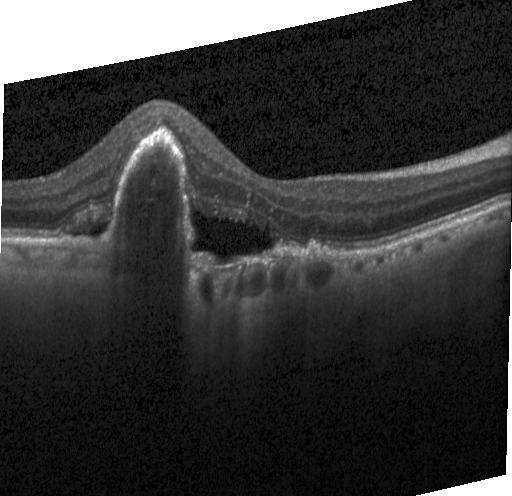 Horizontal scan through the fovea. Spectral-domain optical coherence tomography. Retinal OCT cross-section. Heidelberg Spectralis OCT system
CNV.